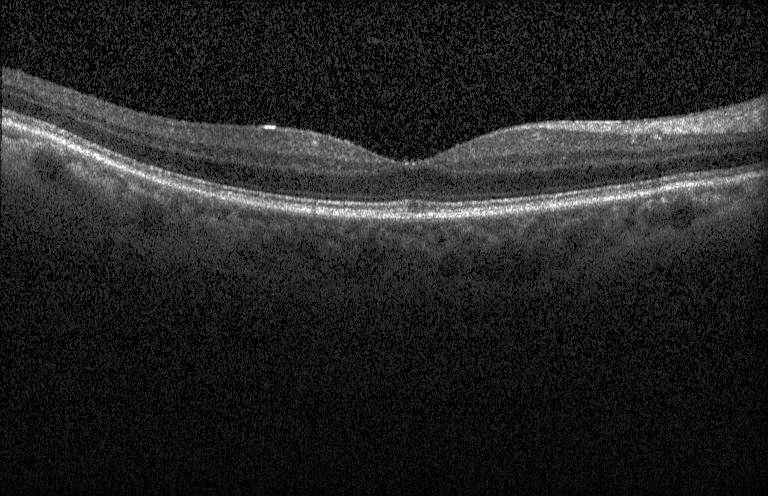

Impression: neither CNV, DME, nor drusen.